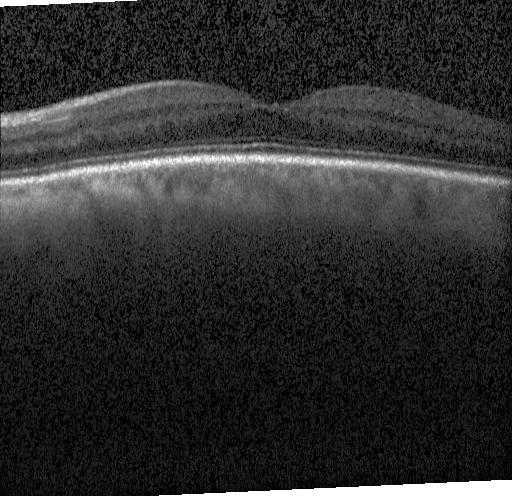
Optical coherence tomography scan
Dx: no choroidal neovascularization, diabetic macular edema, or drusen.